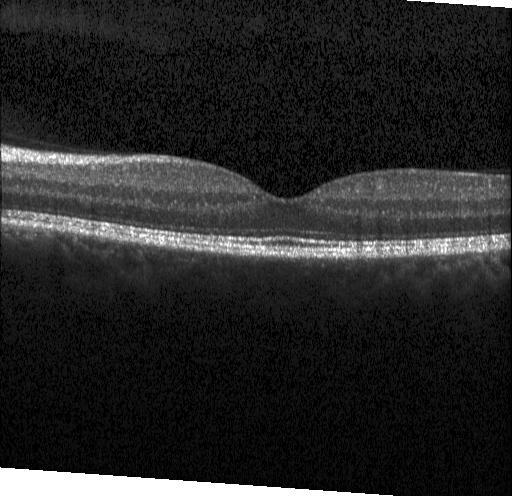 Instrument: Heidelberg Spectralis · optical coherence tomography scan · SD-OCT
Assessment: no CNV, DME, or drusen.